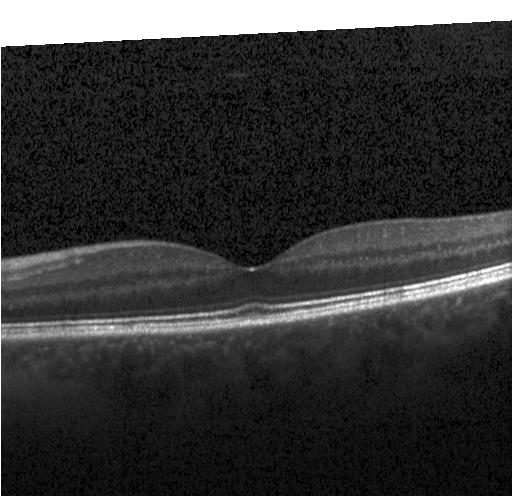 Macular scan. Acquired on a Heidelberg Spectralis. Spectral-domain OCT. Optical coherence tomography scan
Assessment: no choroidal neovascularization, diabetic macular edema, or drusen.